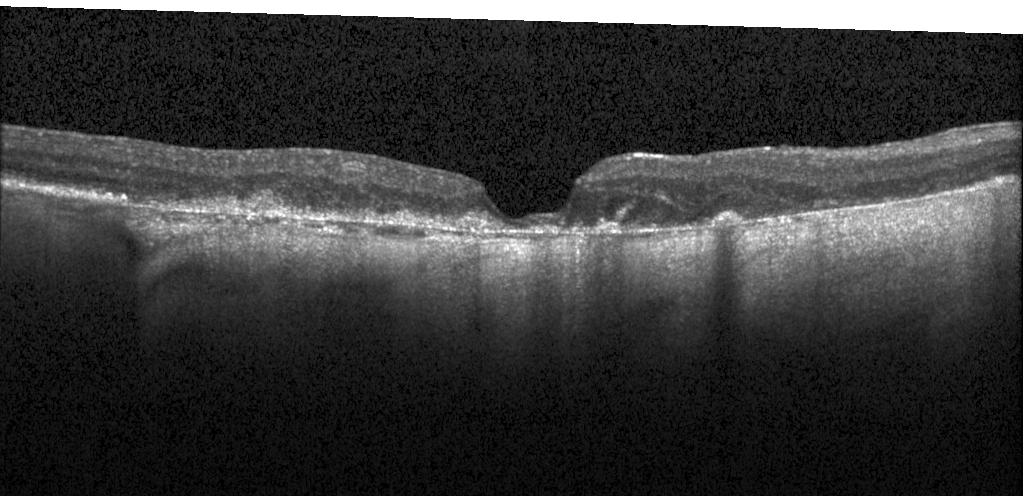 Spectral-domain OCT; retinal OCT B-scan; macular scan. Assessment: a choroidal neovascular membrane.